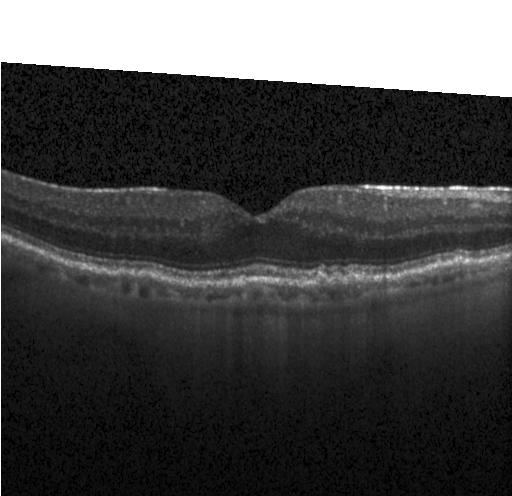 Optical coherence tomography scan. OCT finding: drusen.